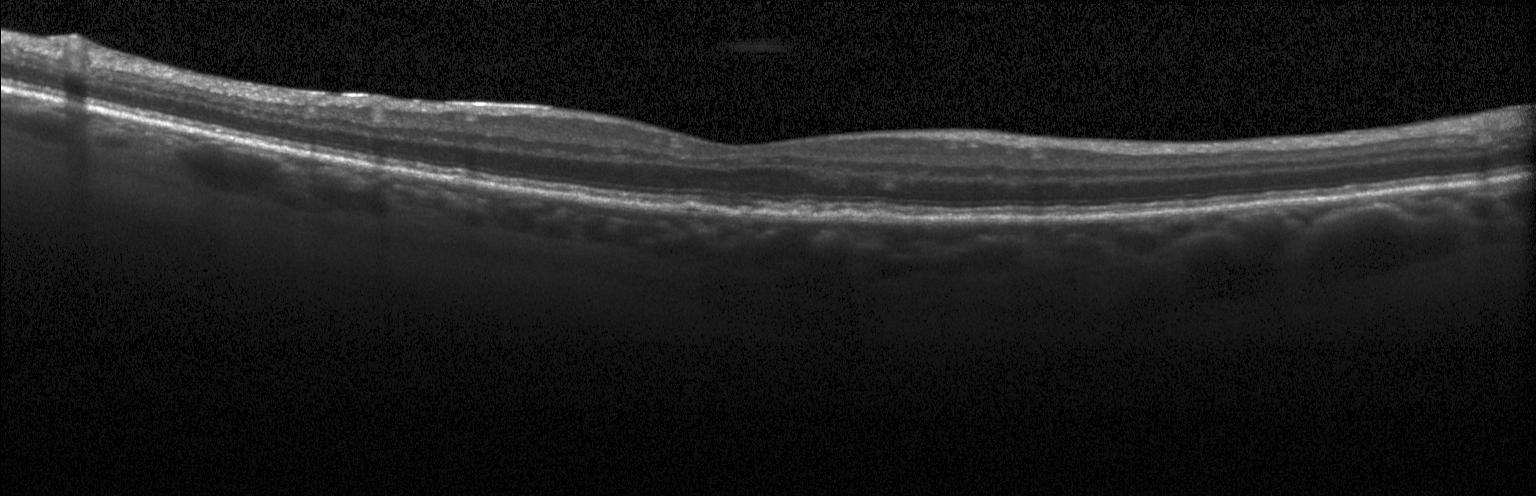
Macular OCT: sub-RPE drusenoid deposits.